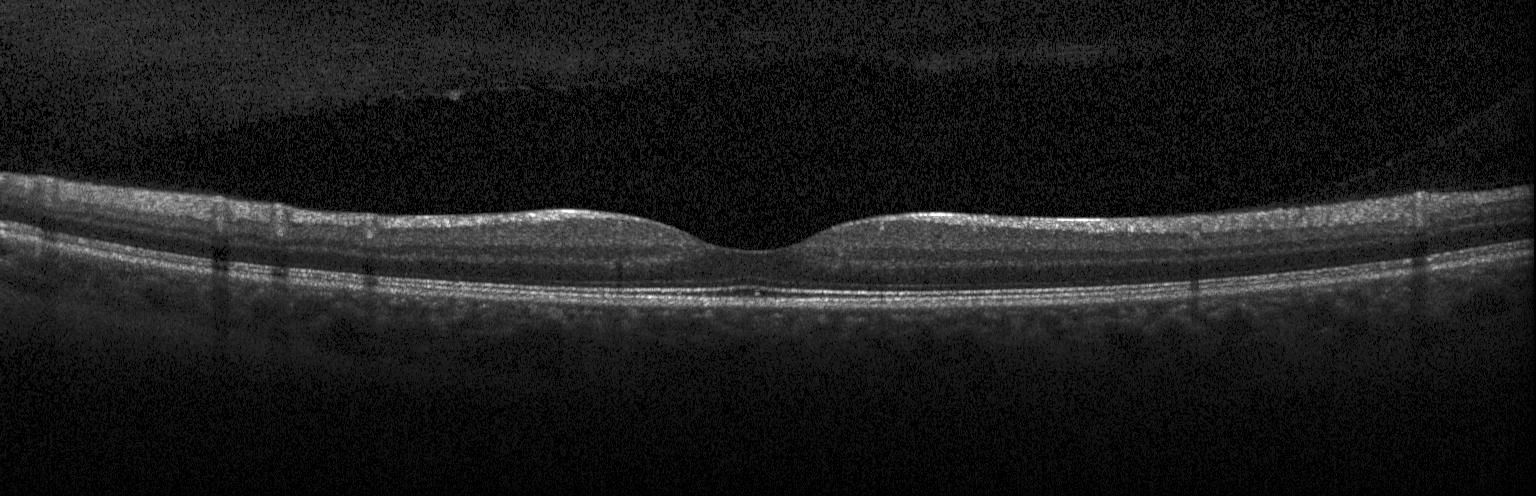 Retinal OCT cross-section
Diagnosis: no choroidal neovascularization, no diabetic macular edema, and no drusen.